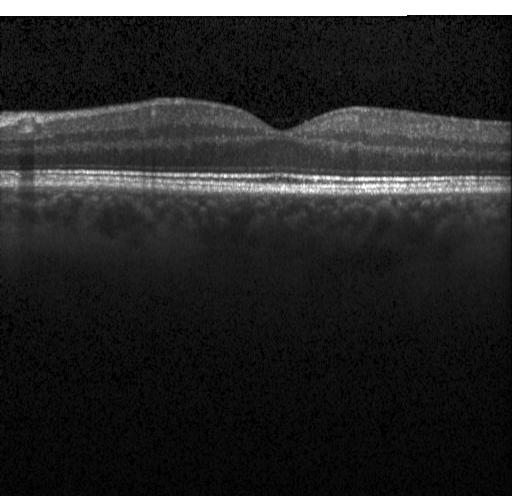

Retinal OCT B-scan · SD-OCT.
This B-scan demonstrates no CNV, DME, or drusen.